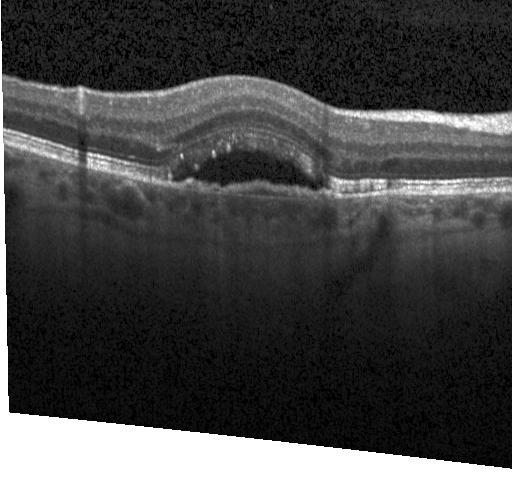

Retinal OCT cross-section · spectral-domain OCT. OCT finding: a choroidal neovascular membrane.